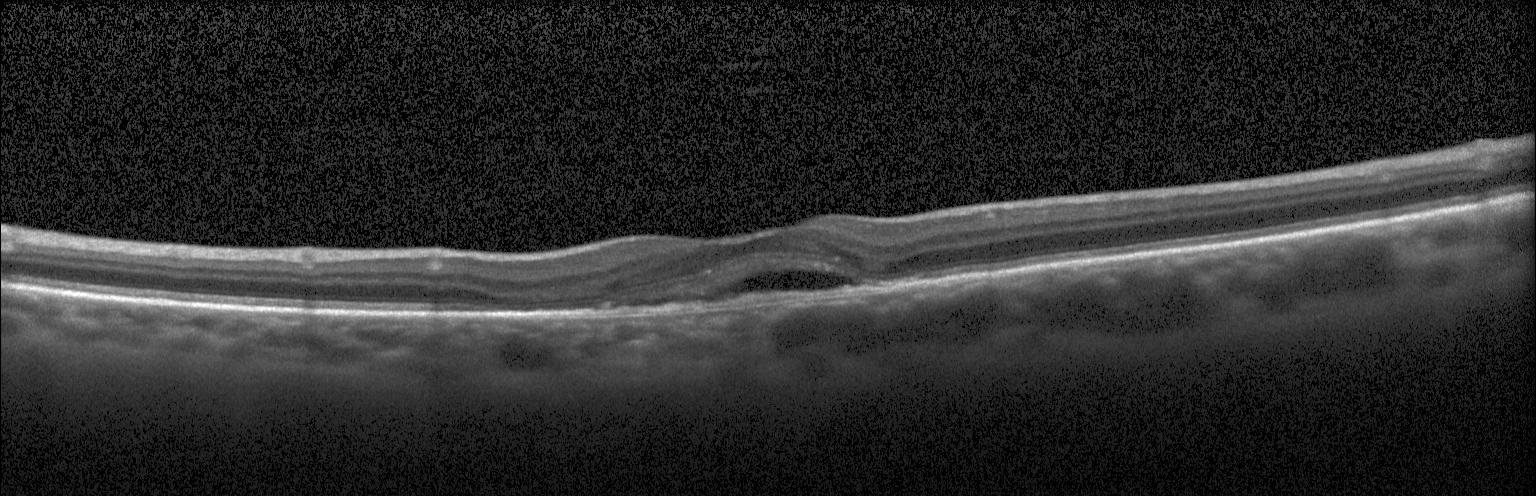
Impression: choroidal neovascularization.